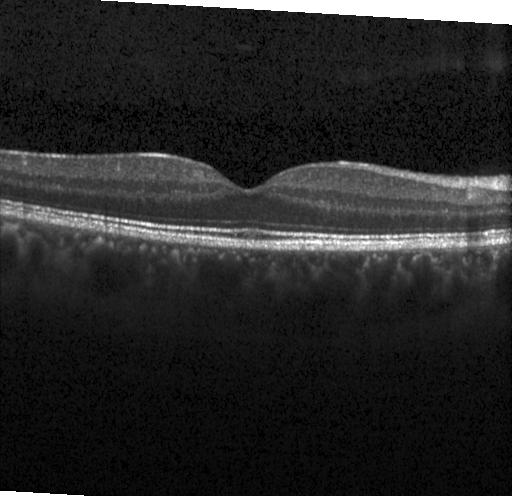
Assessment: neither CNV, DME, nor drusen.